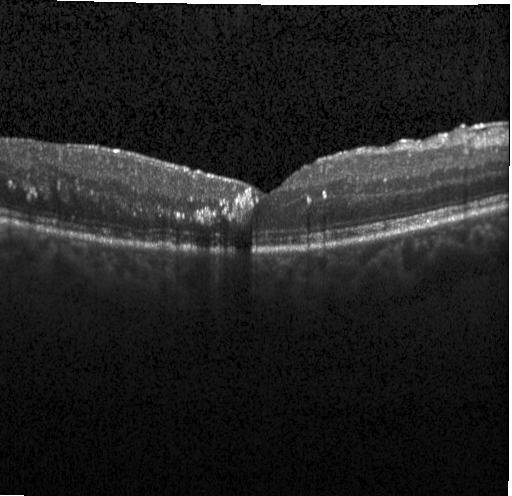
The scan shows diabetic macular edema (DME).